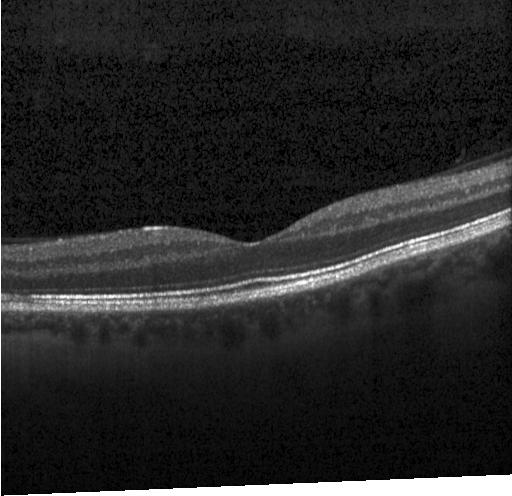 Optical coherence tomography B-scan
Dx: neither choroidal neovascularization, diabetic macular edema, nor drusen.